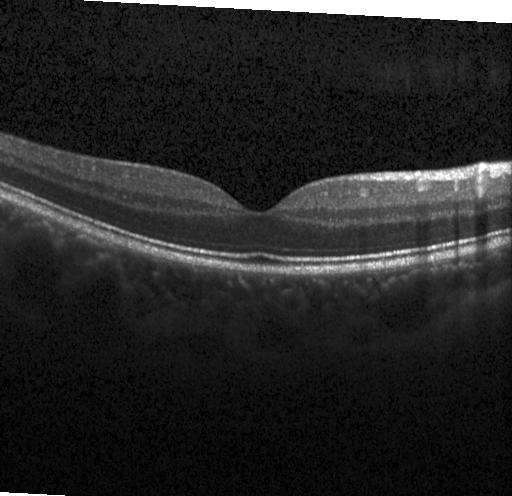 This B-scan demonstrates no CNV, no DME, and no drusen.